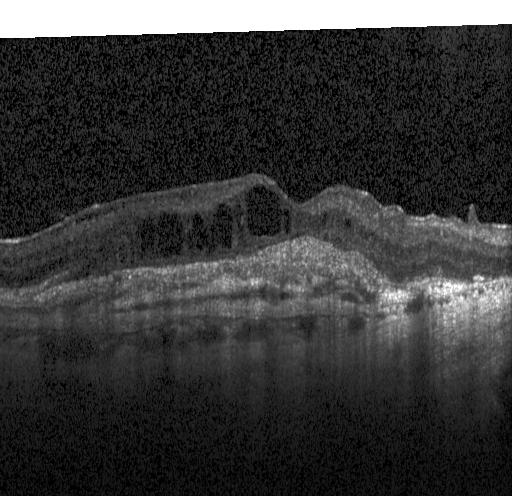 Diagnosis: choroidal neovascularization.